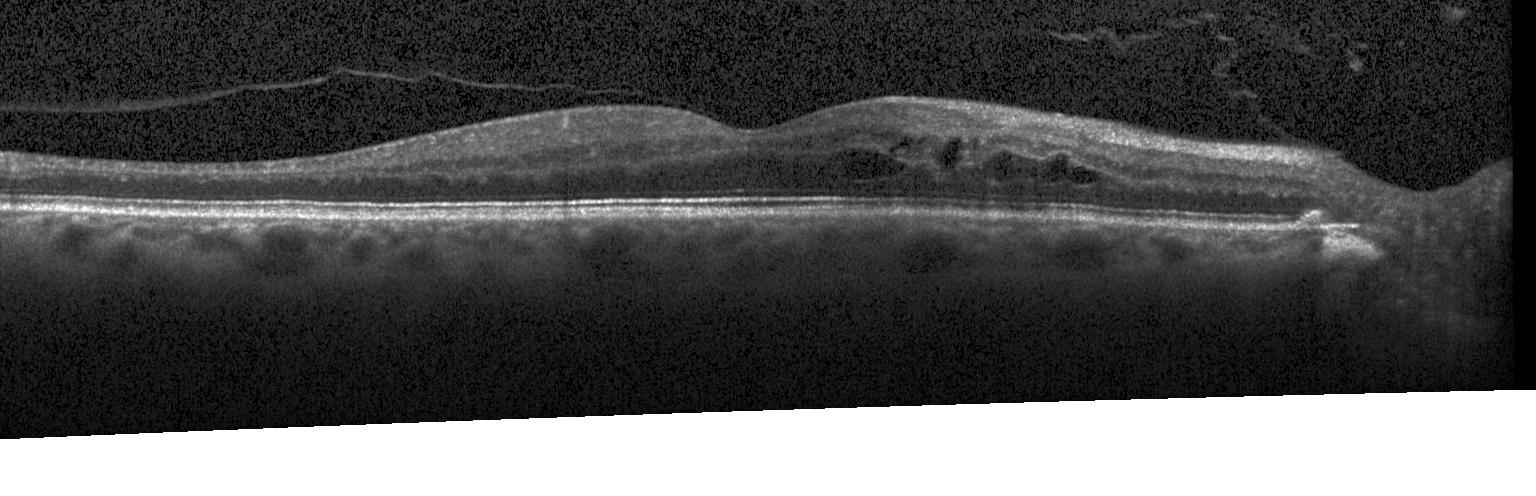 OCT finding: diabetic macular edema (DME).